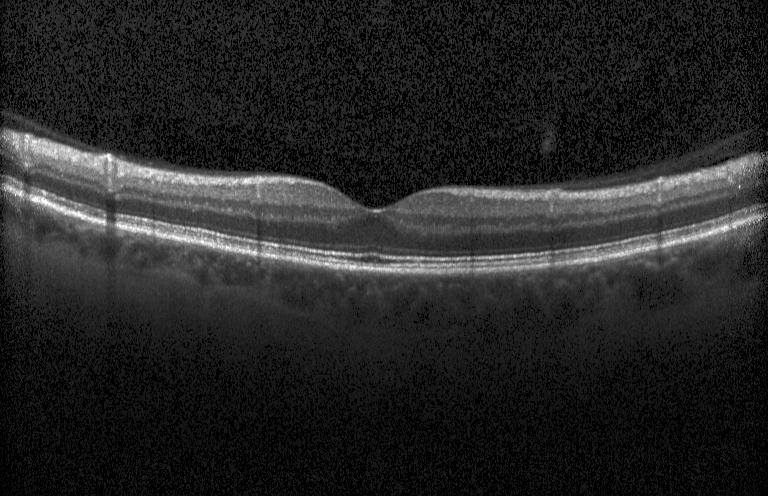

Optical coherence tomography B-scan
Dx: no CNV, DME, or drusen.